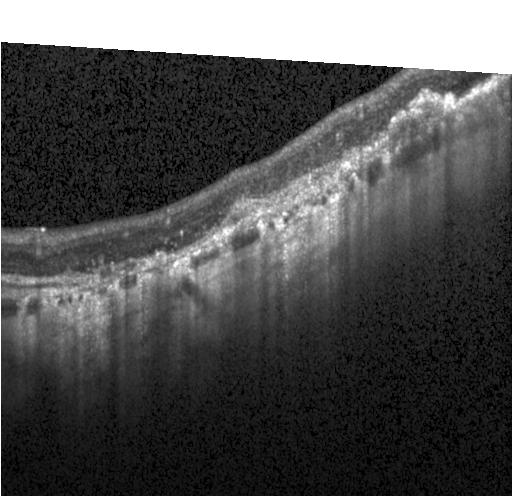
Spectral-domain OCT · optical coherence tomography B-scan — Diagnosis: choroidal neovascularization (CNV).